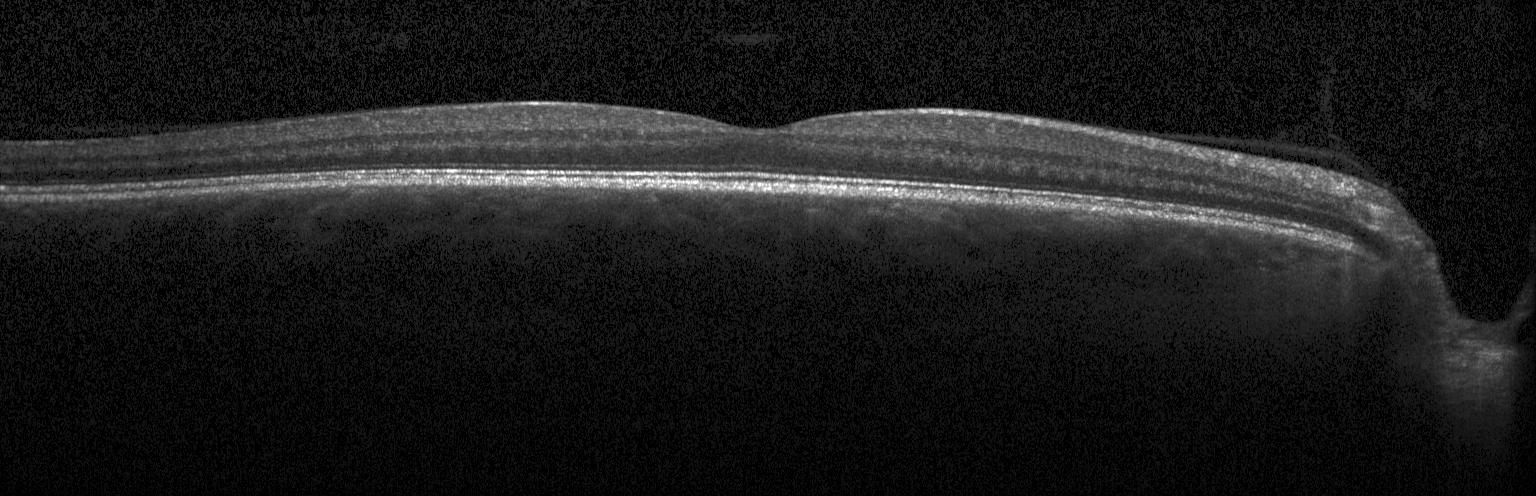
Centered on the fovea; retinal OCT B-scan; spectral-domain optical coherence tomography; instrument: Heidelberg Spectralis.
Assessment: no choroidal neovascularization, diabetic macular edema, or drusen.